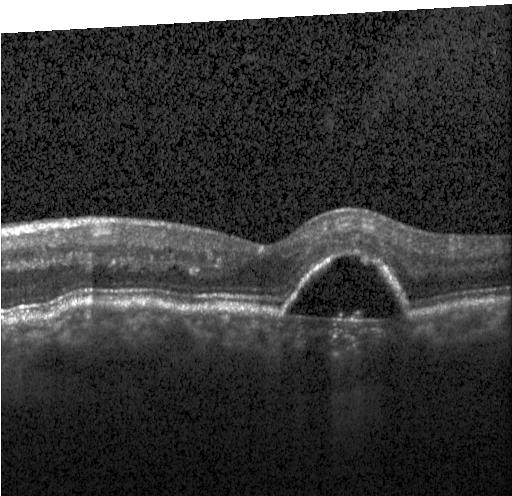

Finding: choroidal neovascularization (CNV).